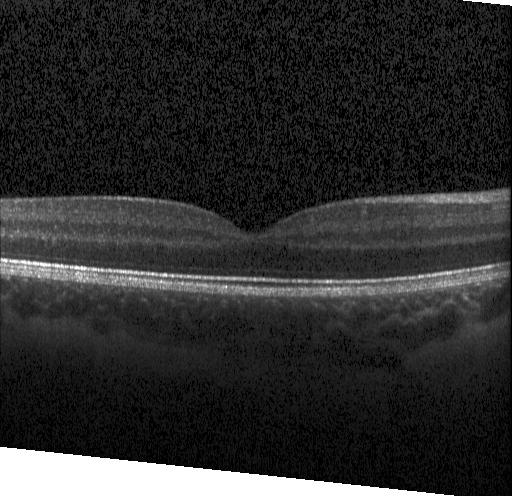 Acquired on a Heidelberg Spectralis. Fovea-centered. Optical coherence tomography scan — Impression: no choroidal neovascularization, no diabetic macular edema, and no drusen.